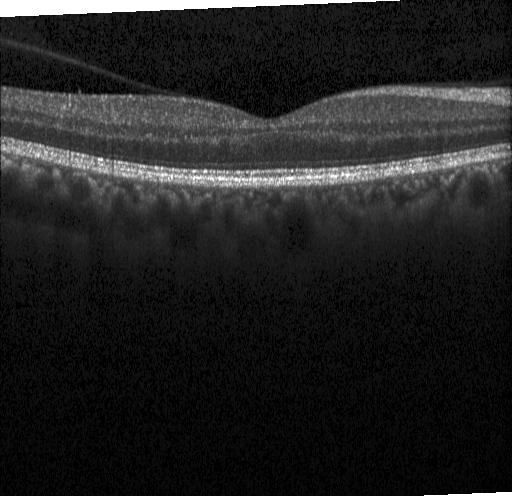
Spectral-domain optical coherence tomography. Through the macula. Acquired on a Heidelberg Spectralis. OCT line scan. Dx: no CNV, DME, or drusen.